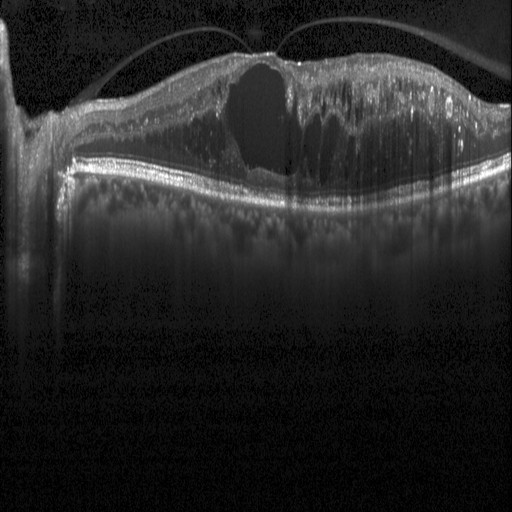
Dx: DME.